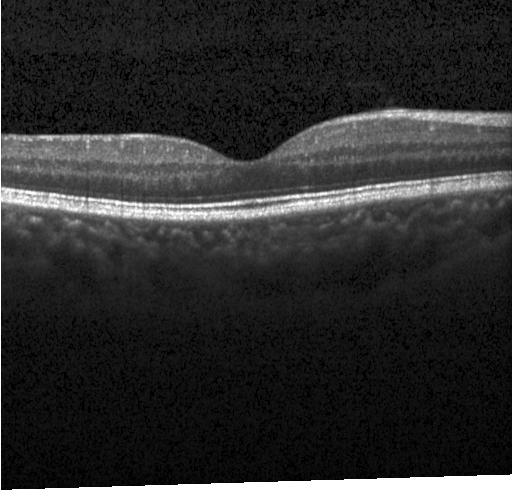
Macular OCT: no choroidal neovascularization, diabetic macular edema, or drusen.